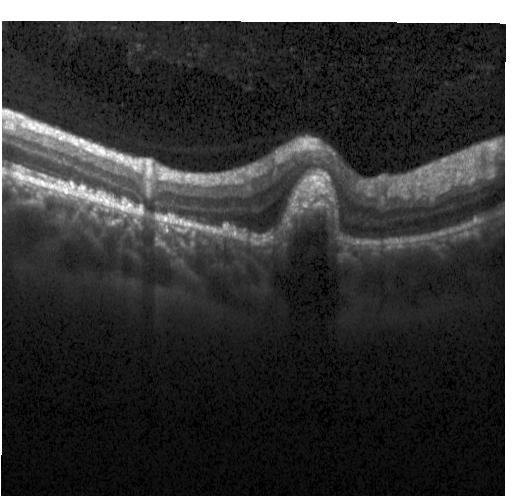 Retinal OCT B-scan
A choroidal neovascular membrane.